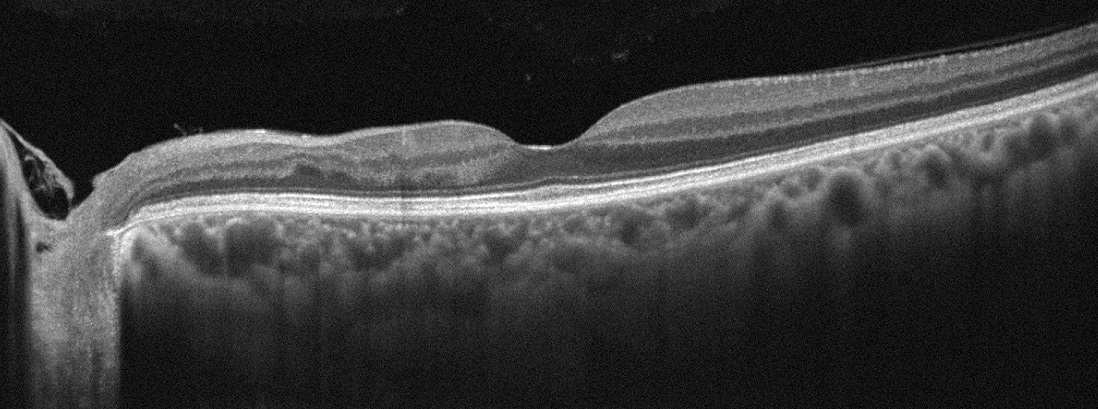 Macular scan. Retinal OCT B-scan. The scan shows retinal vein occlusion (RVO).